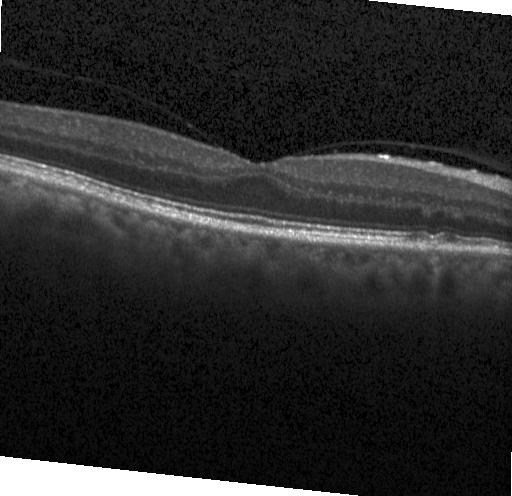 Retinal OCT cross-section showing drusen.